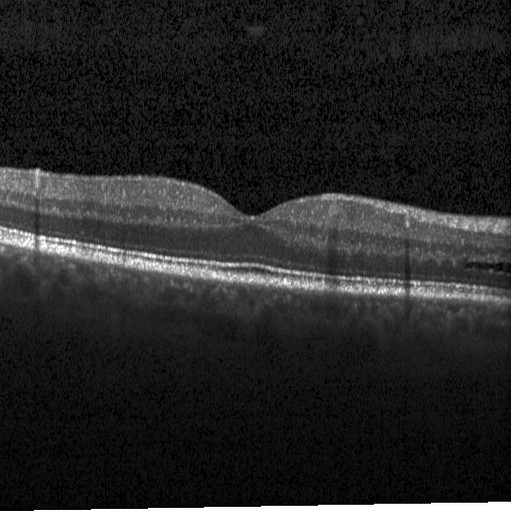 Heidelberg Spectralis OCT system, SD-OCT, optical coherence tomography B-scan — Finding: diabetic macular edema.